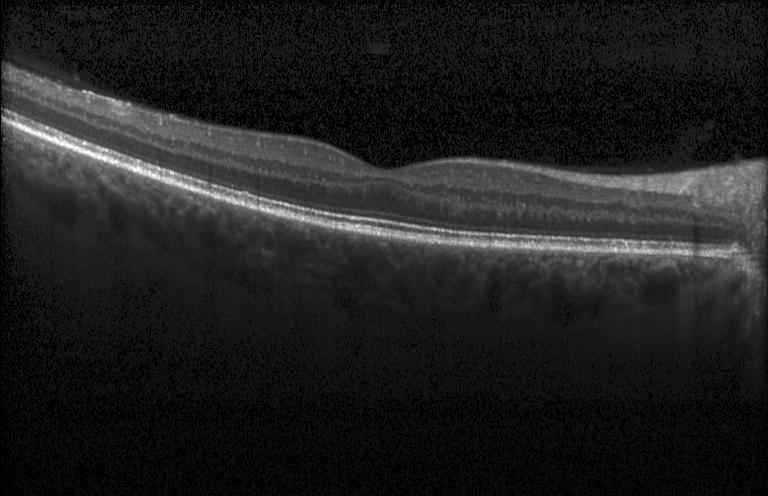 Optical coherence tomography scan · acquired on a Heidelberg Spectralis.
The scan shows neither choroidal neovascularization, diabetic macular edema, nor drusen.